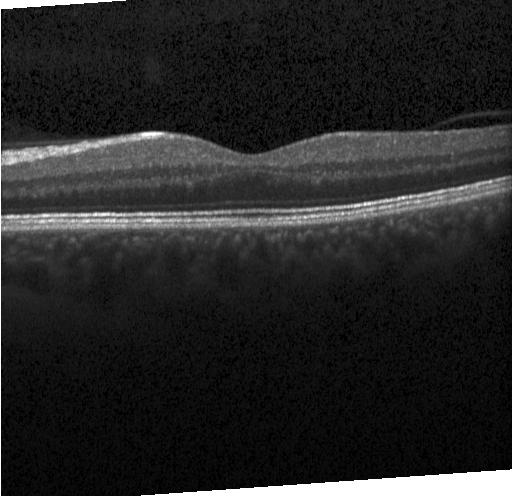
Retinal OCT B-scan
The scan shows no choroidal neovascularization, no diabetic macular edema, and no drusen.